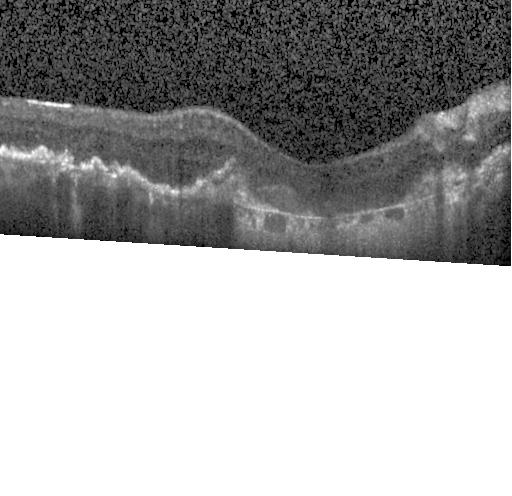
Acquired on a Heidelberg Spectralis; optical coherence tomography scan
Finding: choroidal neovascularization.